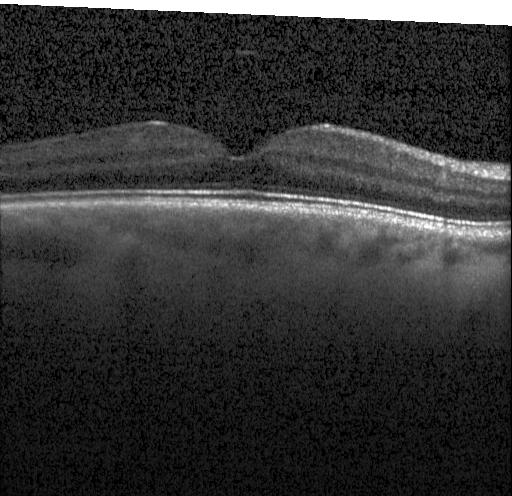

OCT B-scan · spectral-domain OCT · macular scan.
Assessment: no choroidal neovascularization, diabetic macular edema, or drusen.